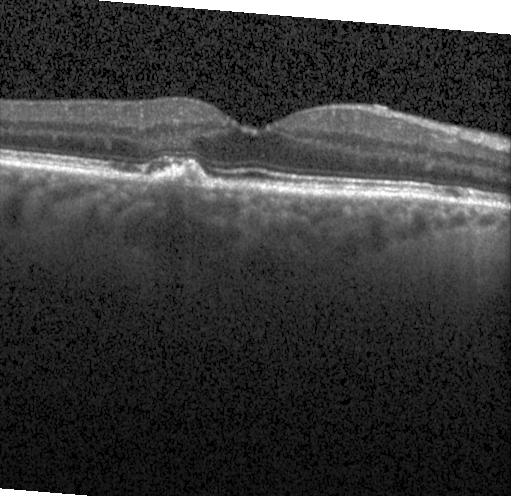
Assessment: a choroidal neovascular membrane.